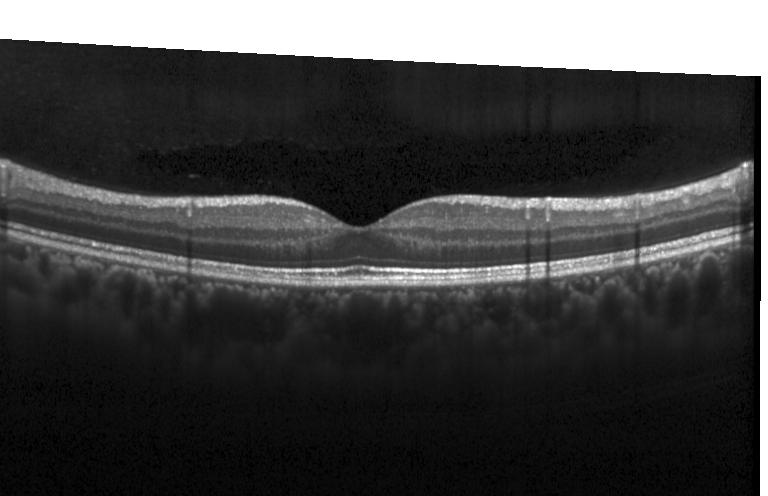

Dx: no CNV, no DME, and no drusen.